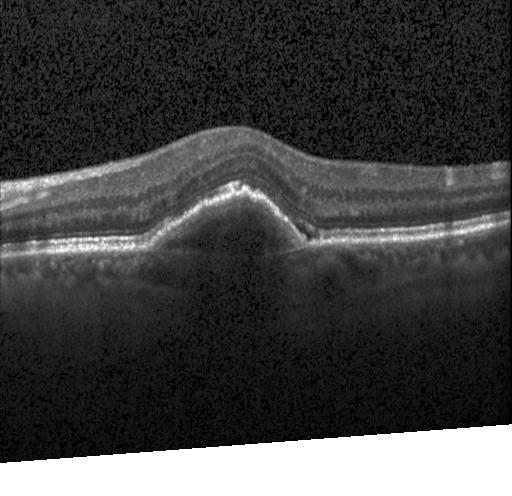
Macular scan, OCT B-scan, Heidelberg Spectralis. The scan shows CNV.